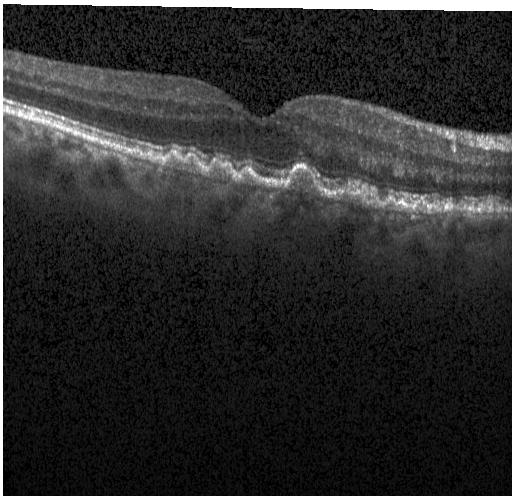

Heidelberg Spectralis; optical coherence tomography scan
Finding: sub-RPE drusenoid deposits.